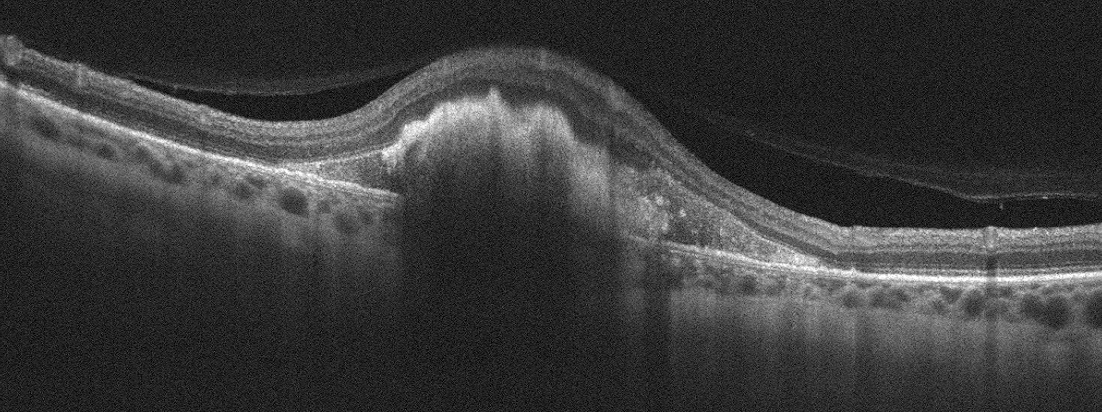
Optical coherence tomography B-scan
Impression: age-related macular degeneration (AMD).